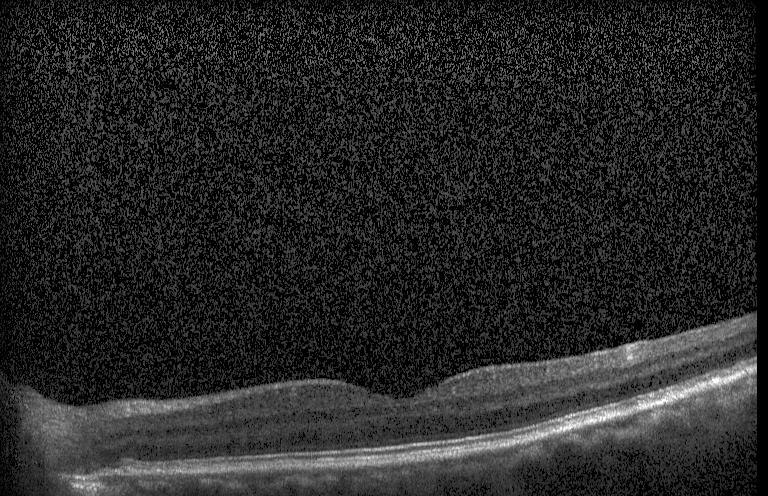 OCT scan showing no CNV, no DME, and no drusen.